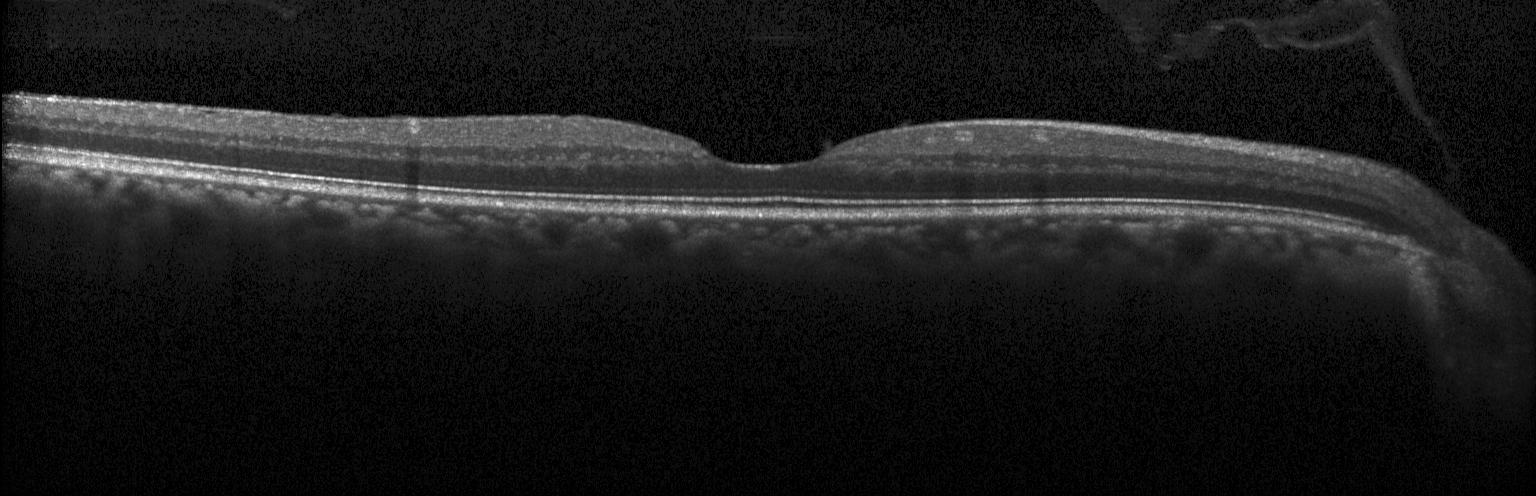
No evidence of choroidal neovascularization, diabetic macular edema, or drusen.